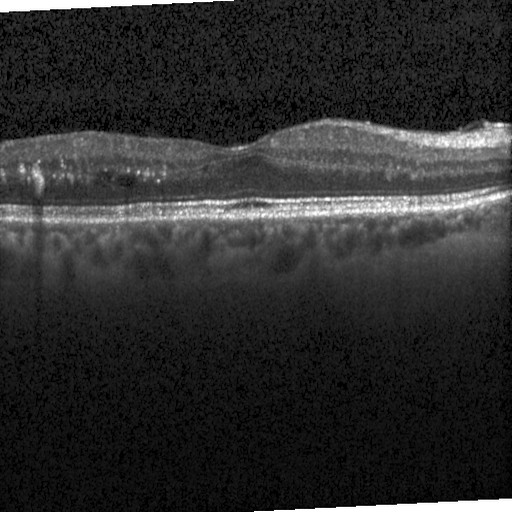
Spectral-domain OCT B-scan: diabetic macular edema.